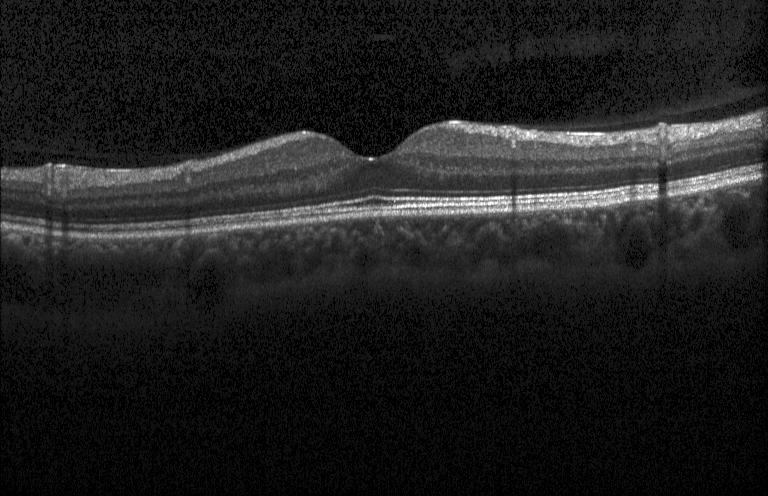 OCT B-scan, horizontal scan through the fovea, spectral-domain optical coherence tomography
Diagnosis: no evidence of choroidal neovascularization, diabetic macular edema, or drusen.